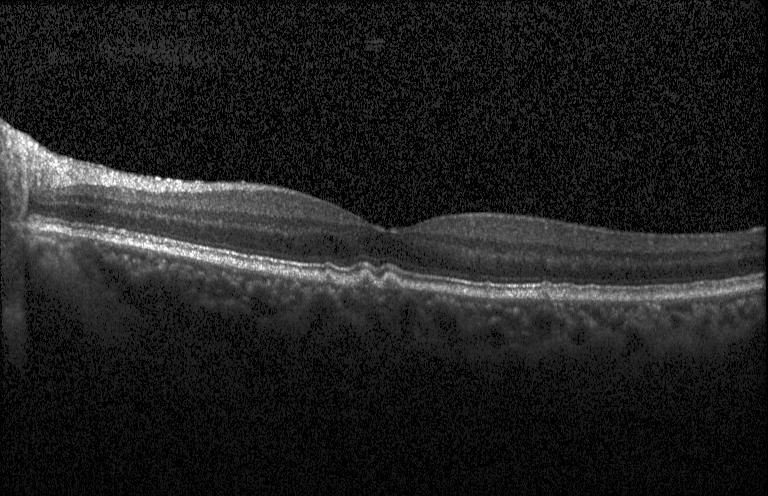

Macular scan · retinal OCT cross-section · Heidelberg Spectralis OCT system
Finding: sub-RPE drusenoid deposits.